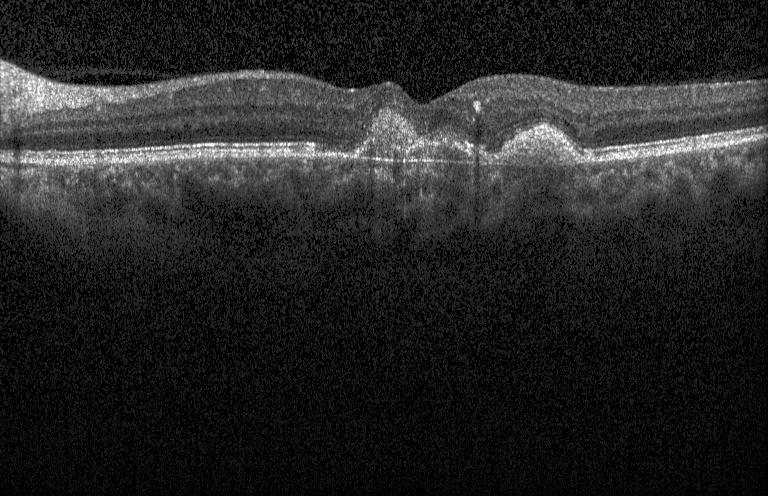 Macular OCT: a choroidal neovascular membrane.